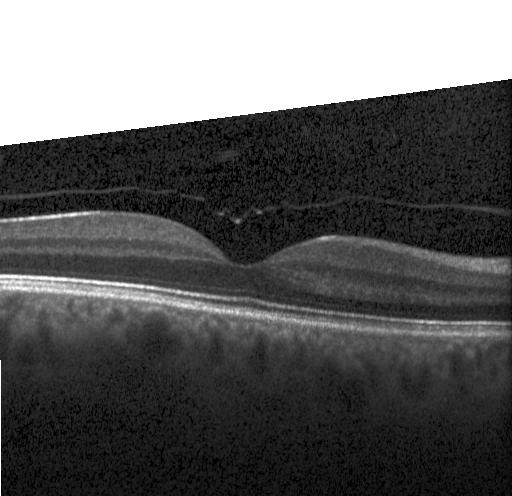
Macular scan · acquired on a Heidelberg Spectralis · optical coherence tomography scan. This B-scan demonstrates no CNV, DME, or drusen.